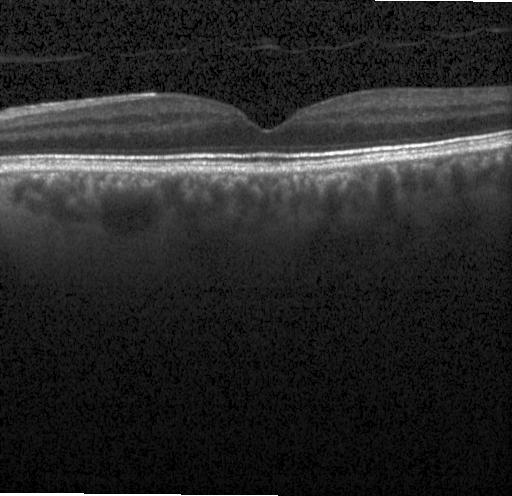 OCT line scan · fovea-centered. OCT finding: no evidence of choroidal neovascularization, diabetic macular edema, or drusen.